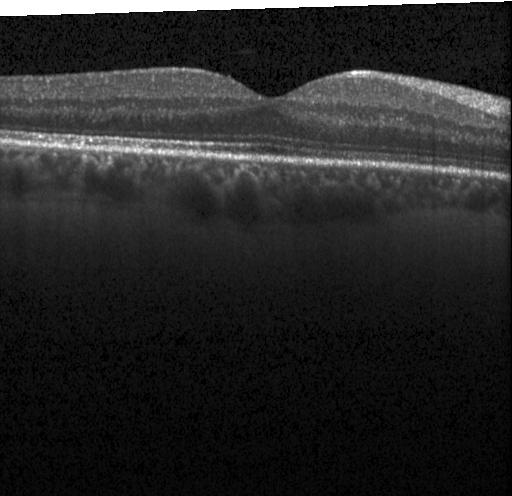

OCT line scan · Heidelberg Spectralis — Diagnosis: neither choroidal neovascularization, diabetic macular edema, nor drusen.